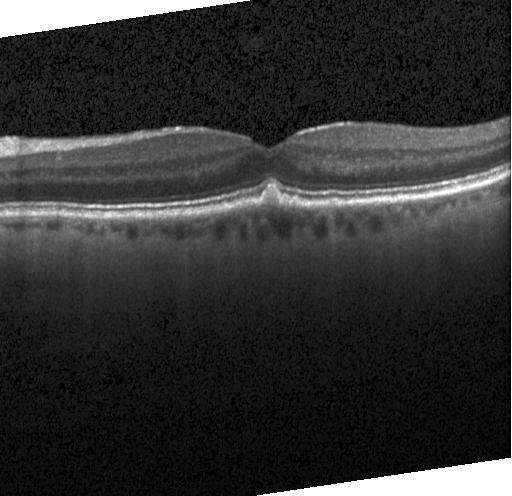
OCT finding: drusen.